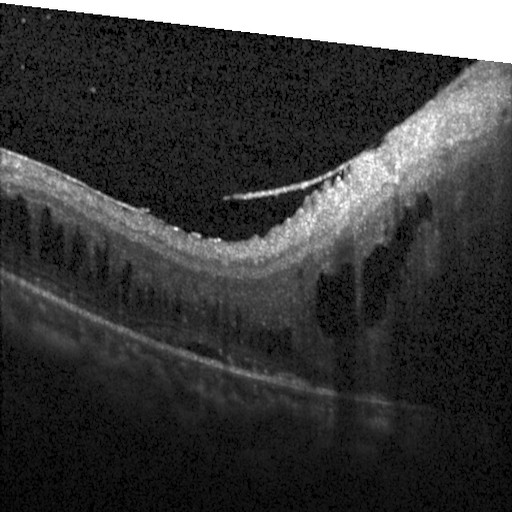

Spectral-domain OCT B-scan: DME.